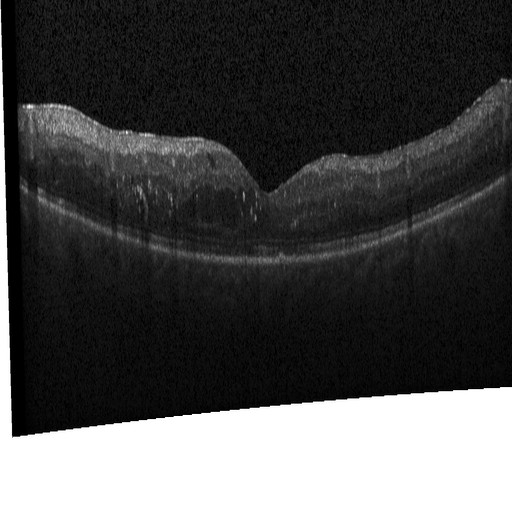

Spectral-domain OCT. Optical coherence tomography B-scan. Acquired on a Heidelberg Spectralis. Fovea-centered — Diagnosis: diabetic macular edema (DME).